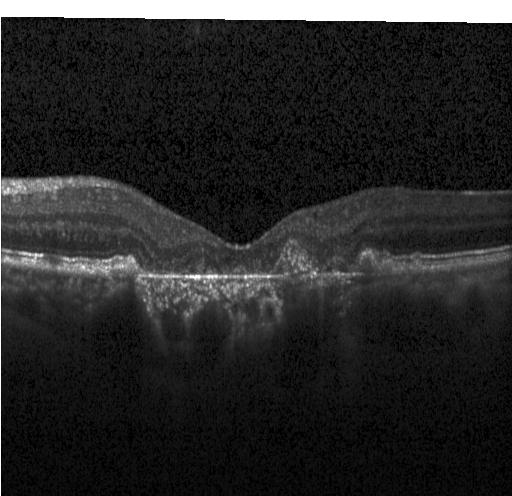

Retinal OCT cross-section. Macular scan. Spectral-domain OCT. Heidelberg Spectralis. Finding: CNV.